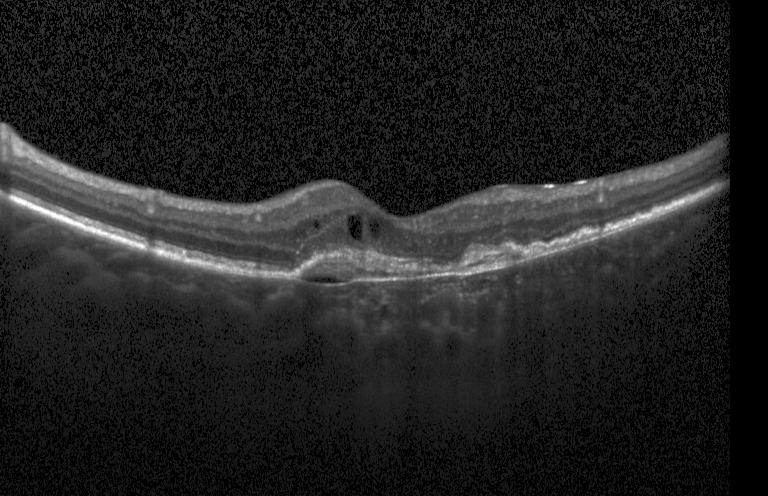
Heidelberg Spectralis OCT system; optical coherence tomography scan. Impression: choroidal neovascularization (CNV).